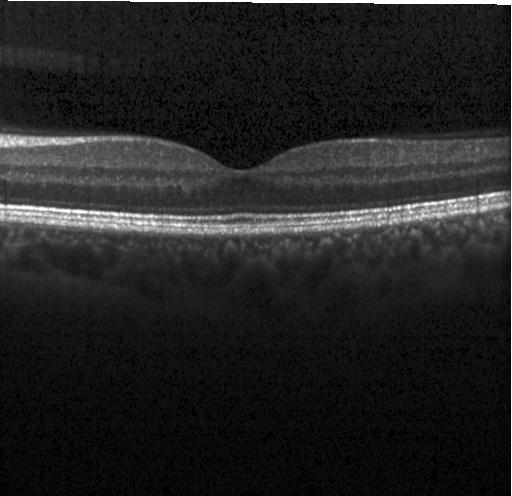

Optical coherence tomography B-scan · horizontal scan through the fovea — Macular OCT: no evidence of CNV, DME, or drusen.